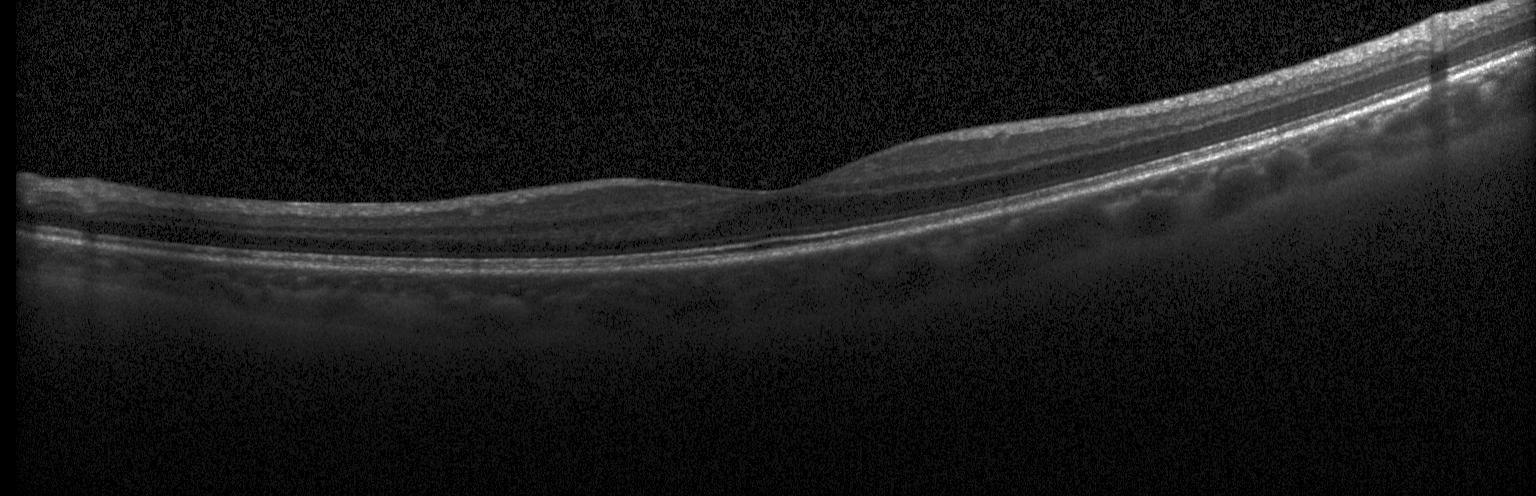

Impression: neither choroidal neovascularization, diabetic macular edema, nor drusen.